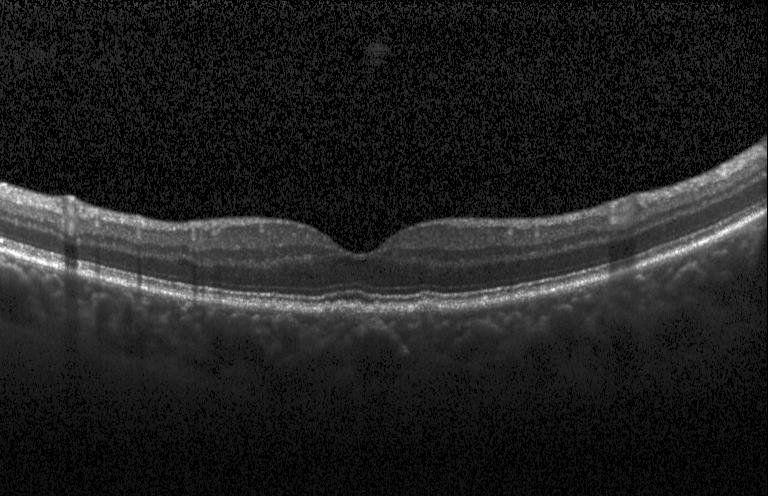
OCT line scan
Diagnosis: sub-RPE drusenoid deposits.